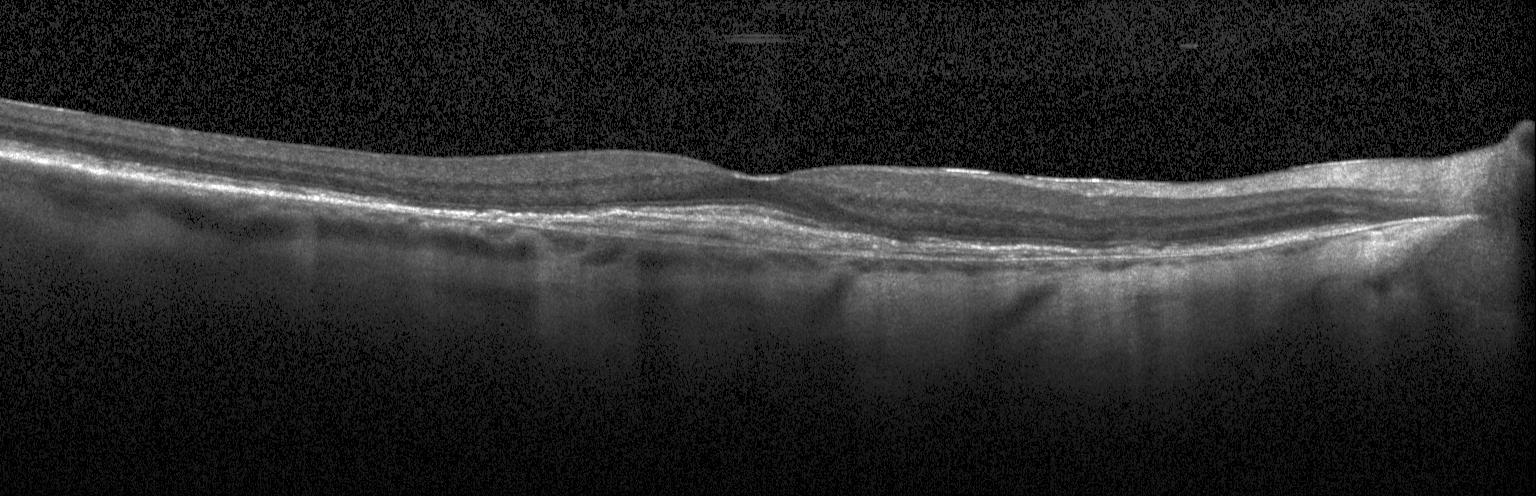

Macular OCT: a choroidal neovascular membrane.